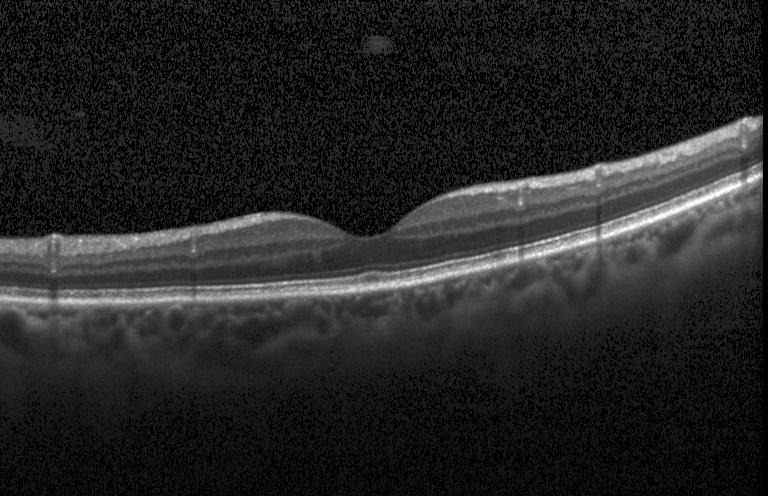
No evidence of choroidal neovascularization, diabetic macular edema, or drusen.